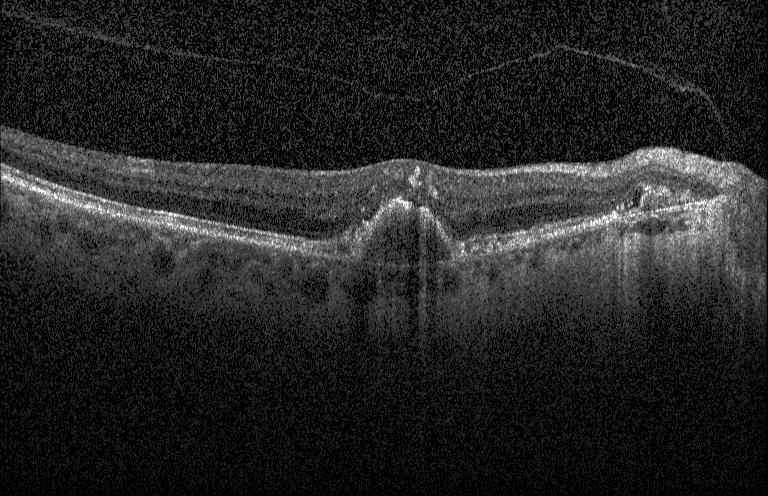 OCT line scan — Impression: choroidal neovascularization.